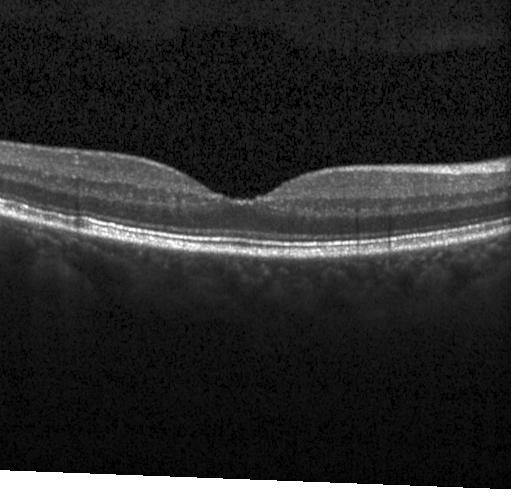
No CNV, DME, or drusen.